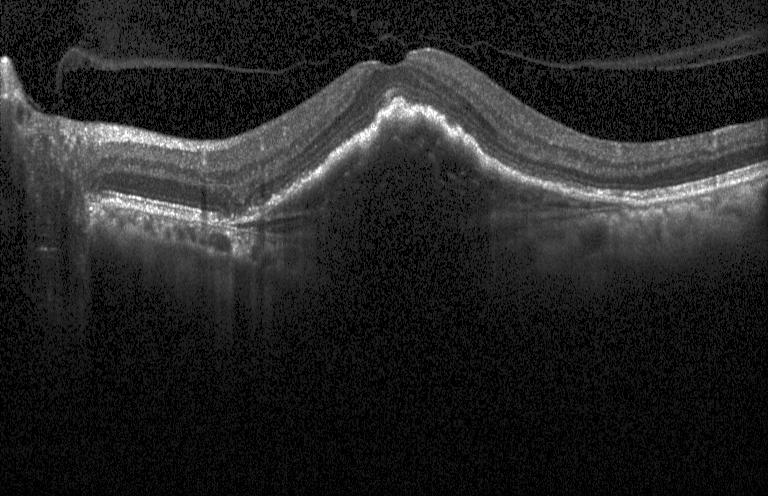
Acquired on a Heidelberg Spectralis · retinal OCT B-scan. Assessment: choroidal neovascularization.